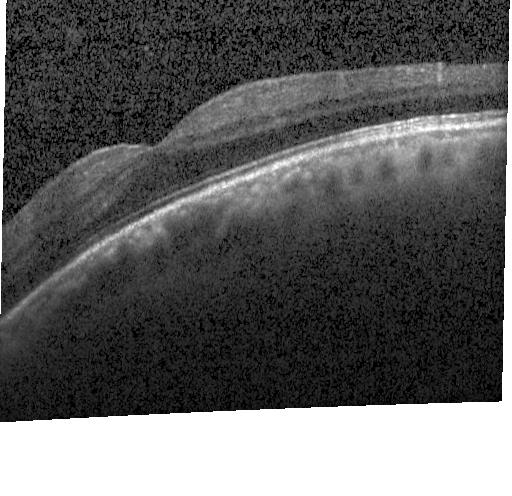
Spectral-domain OCT. Horizontal scan through the fovea. Heidelberg Spectralis OCT system. Retinal OCT cross-section. Assessment: no evidence of choroidal neovascularization, diabetic macular edema, or drusen.